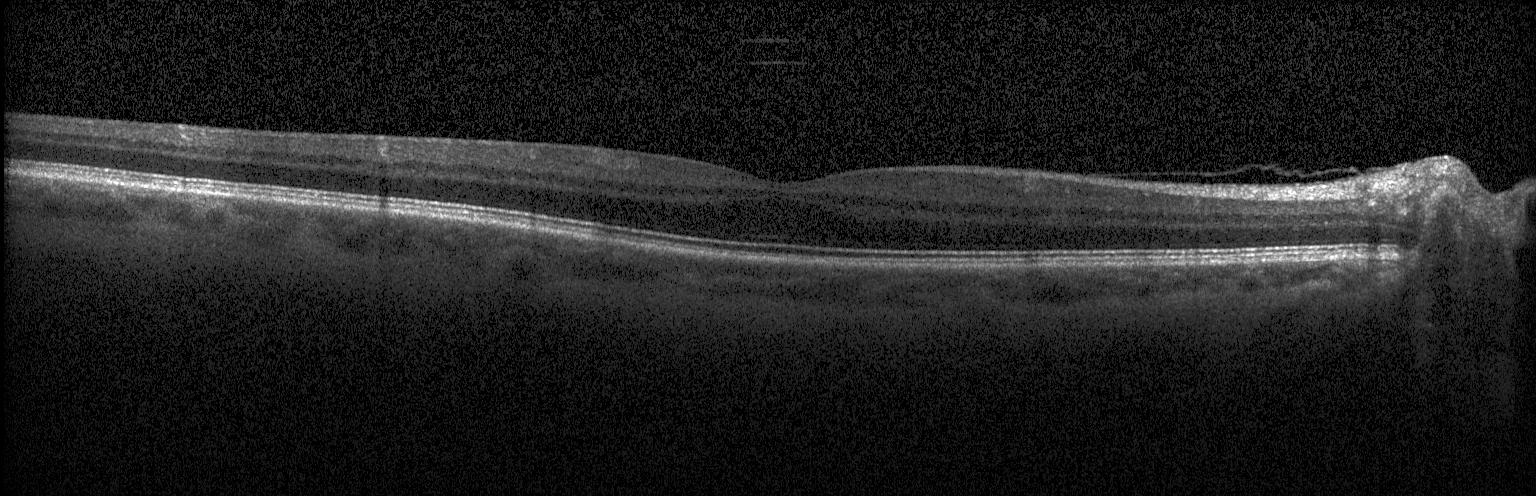 Spectral-domain OCT B-scan: no evidence of choroidal neovascularization, diabetic macular edema, or drusen.